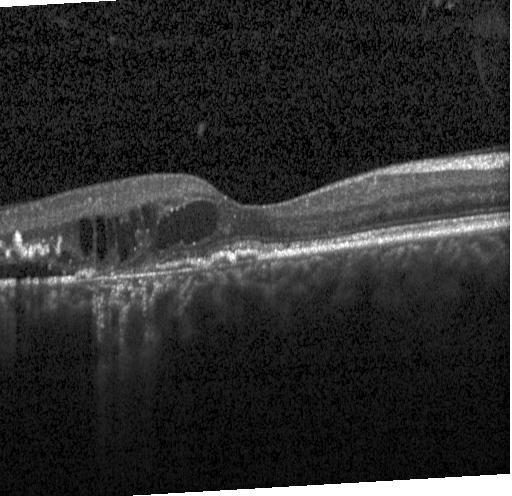
Through the macula · OCT B-scan.
Diagnosis: choroidal neovascularization.